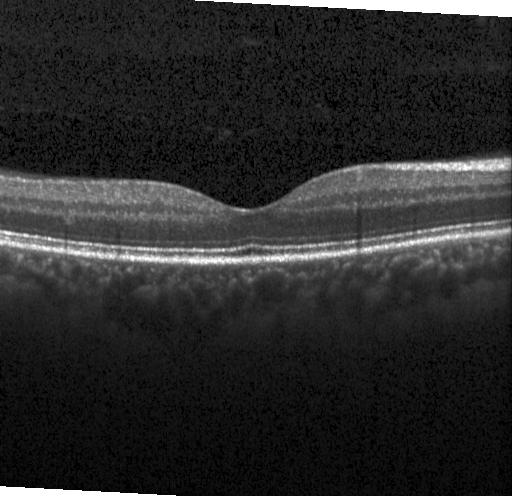

OCT line scan · Heidelberg Spectralis OCT system. Macular OCT: no choroidal neovascularization, diabetic macular edema, or drusen.